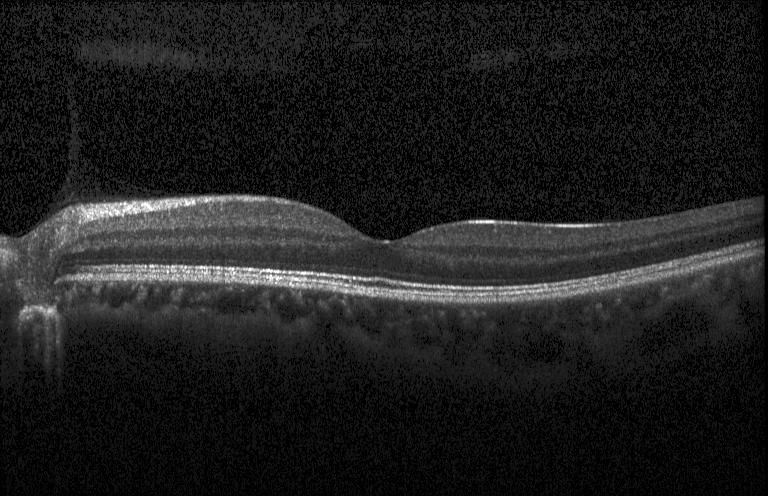
Macular OCT: no evidence of choroidal neovascularization, diabetic macular edema, or drusen.